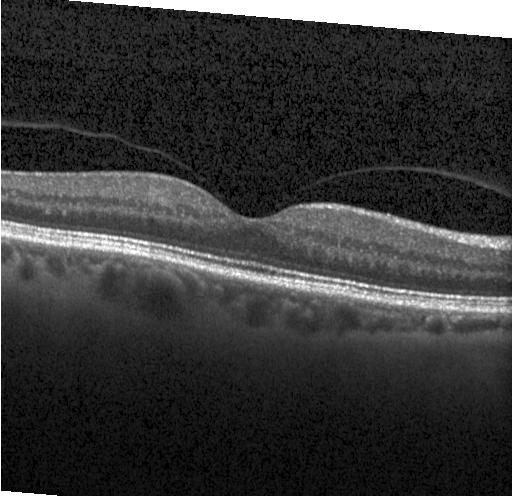
Diagnosis: neither CNV, DME, nor drusen.